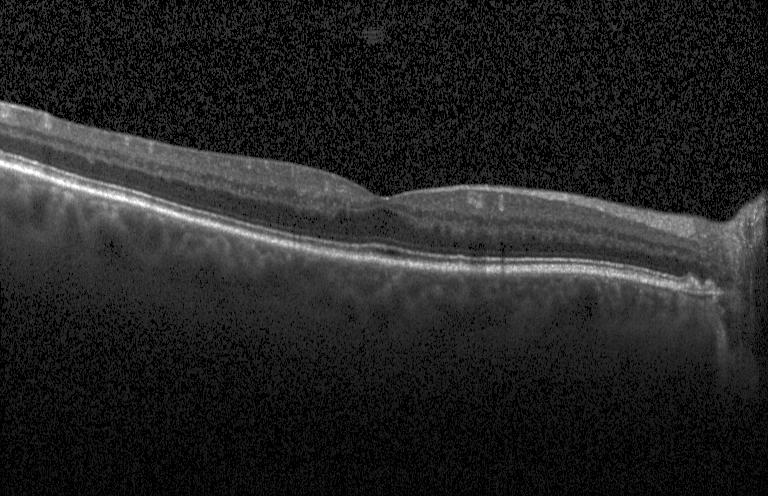

Through the macula · optical coherence tomography B-scan · SD-OCT · Heidelberg Spectralis — The scan shows no CNV, DME, or drusen.